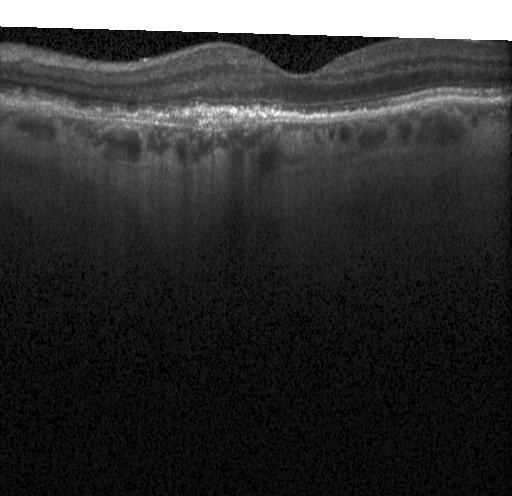 OCT line scan, centered on the fovea, Heidelberg Spectralis OCT system, SD-OCT. OCT finding: choroidal neovascularization.